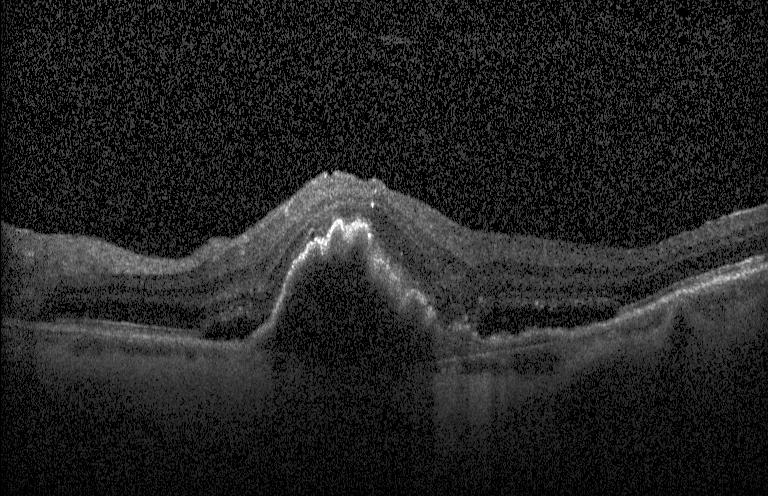
Optical coherence tomography scan — A choroidal neovascular membrane.